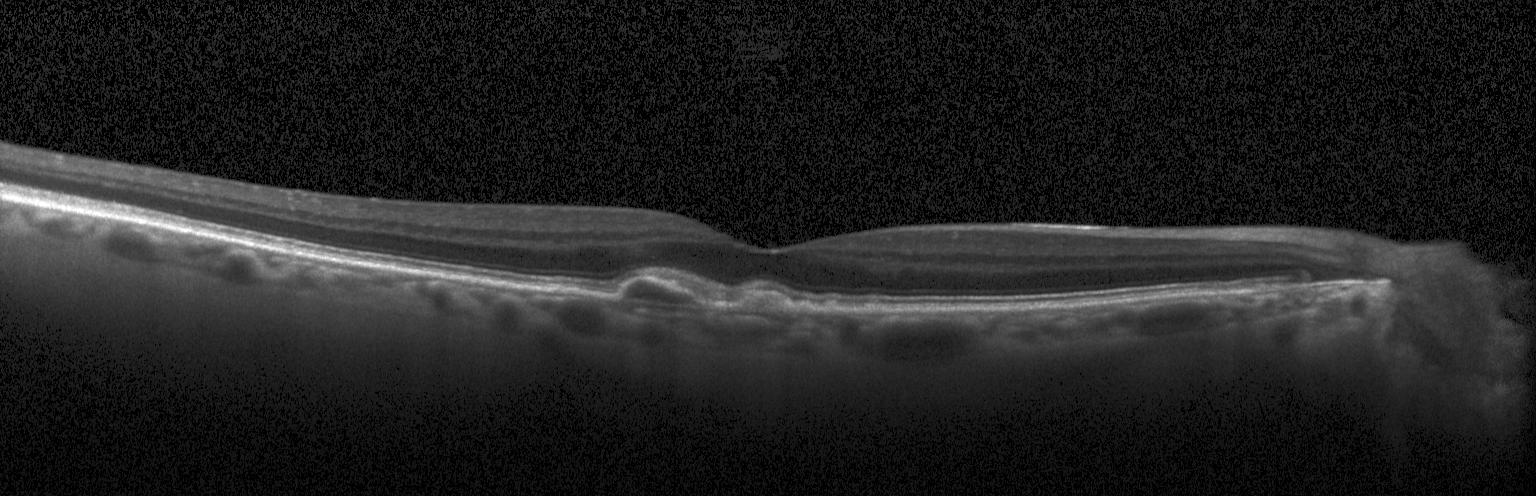
OCT finding: a choroidal neovascular membrane.